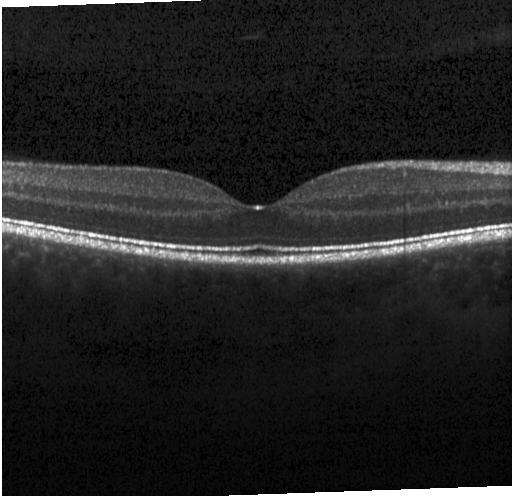
Macular scan · optical coherence tomography scan
Macular OCT: no evidence of choroidal neovascularization, diabetic macular edema, or drusen.